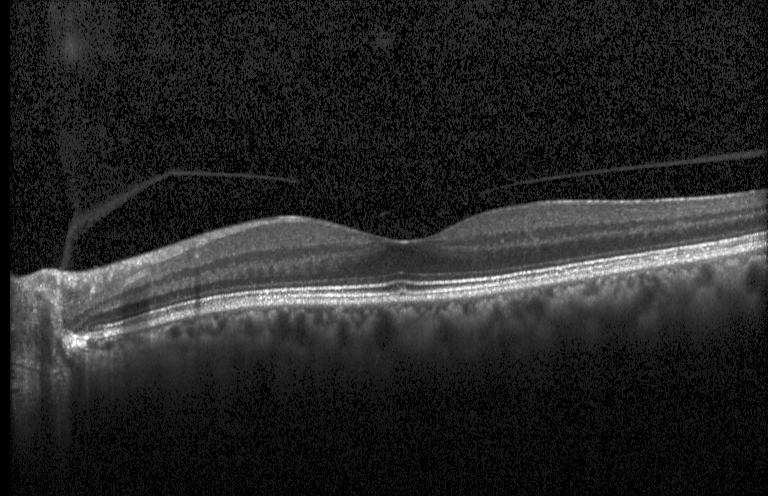
OCT B-scan; Heidelberg Spectralis; fovea-centered — Assessment: no choroidal neovascularization, no diabetic macular edema, and no drusen.